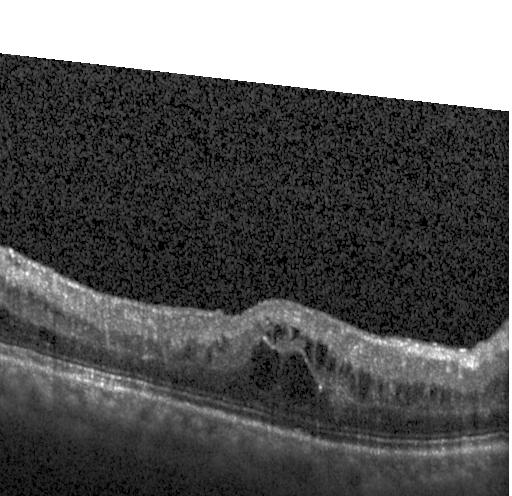
OCT scan showing DME.